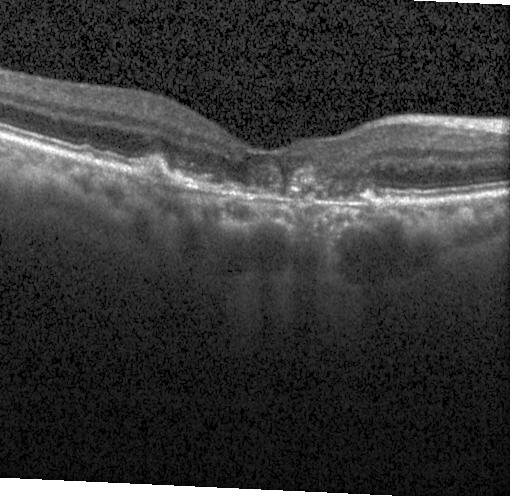

Optical coherence tomography B-scan — This B-scan demonstrates a choroidal neovascular membrane.